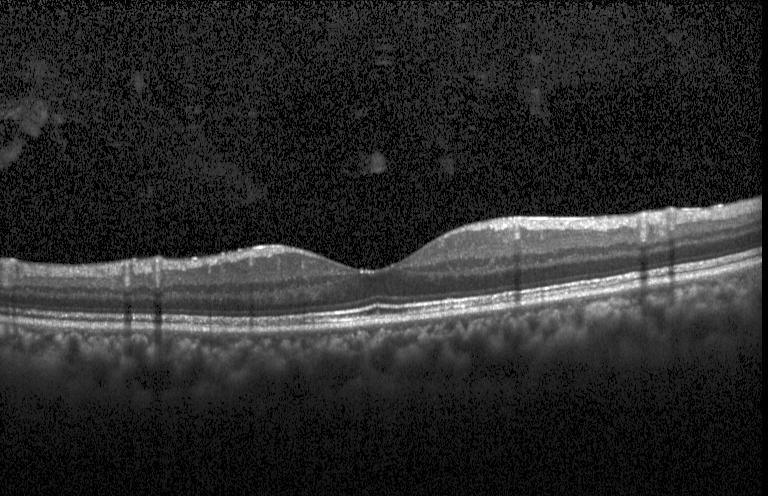

Optical coherence tomography B-scan, Heidelberg Spectralis, fovea-centered, SD-OCT. The scan shows neither choroidal neovascularization, diabetic macular edema, nor drusen.